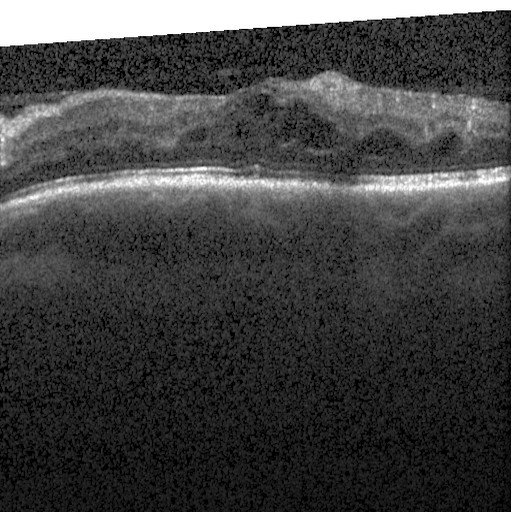 Spectral-domain optical coherence tomography. Retinal OCT B-scan. Heidelberg Spectralis.
Diagnosis: diabetic macular edema (DME).